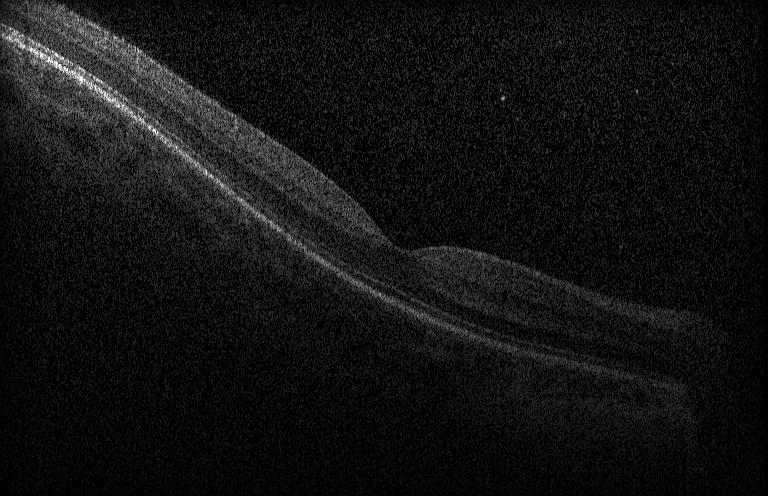
Spectral-domain optical coherence tomography. Through the macula. OCT line scan — Impression: no choroidal neovascularization, diabetic macular edema, or drusen.